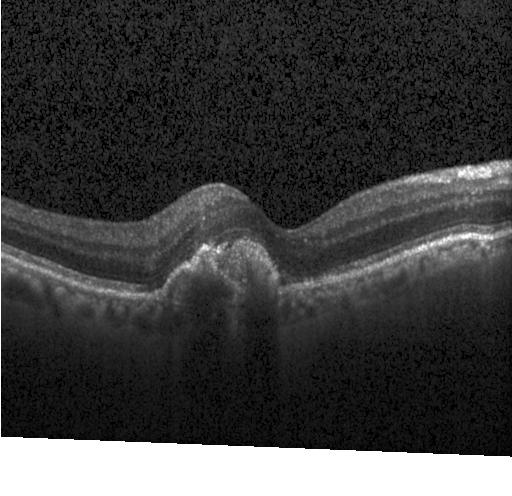

Finding: a choroidal neovascular membrane.